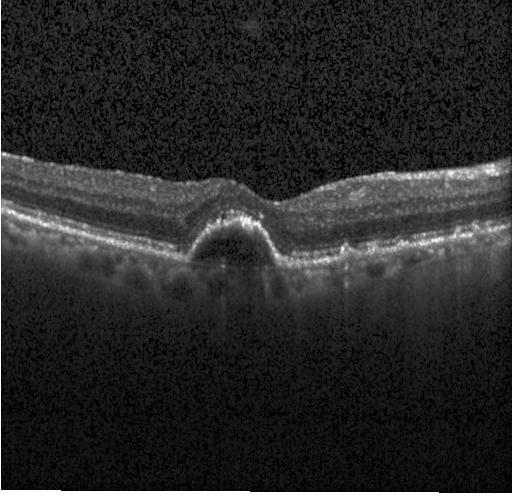 Retinal OCT cross-section showing a choroidal neovascular membrane.